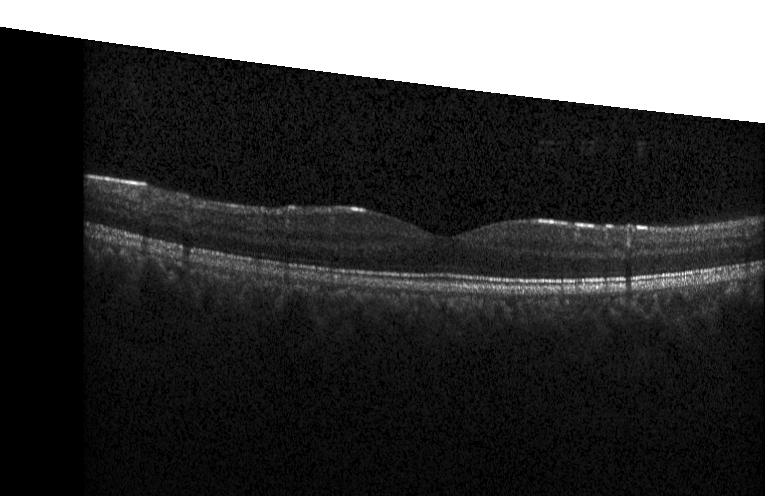
OCT line scan
Finding: neither CNV, DME, nor drusen.